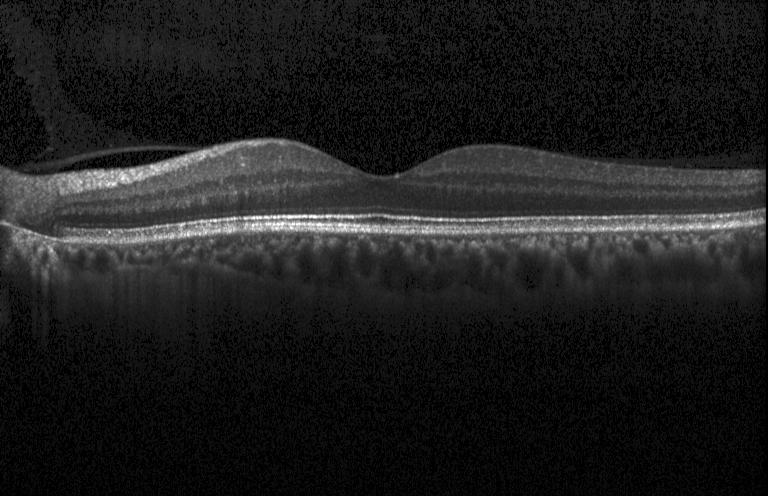
Optical coherence tomography B-scan; acquired on a Heidelberg Spectralis; macular scan; spectral-domain optical coherence tomography. Finding: no choroidal neovascularization, no diabetic macular edema, and no drusen.